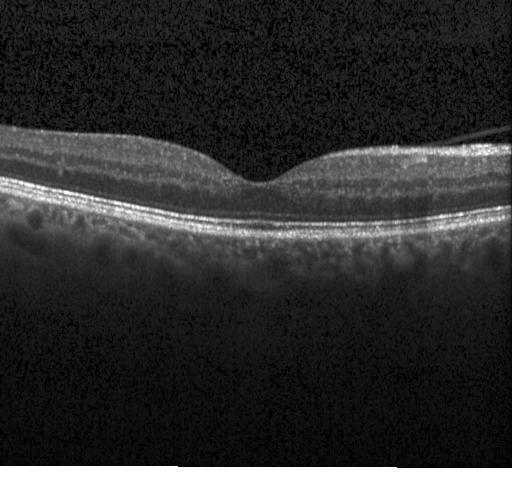 Finding: neither choroidal neovascularization, diabetic macular edema, nor drusen.